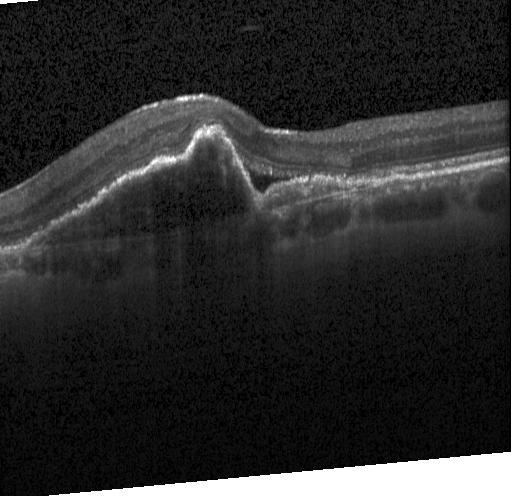 Acquired on a Heidelberg Spectralis · OCT line scan · centered on the fovea. Diagnosis: choroidal neovascularization (CNV).